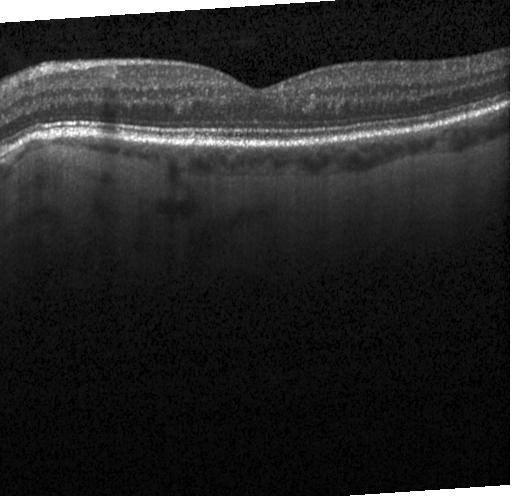
Retinal OCT B-scan. Macular scan. Heidelberg Spectralis OCT system.
This B-scan demonstrates neither choroidal neovascularization, diabetic macular edema, nor drusen.